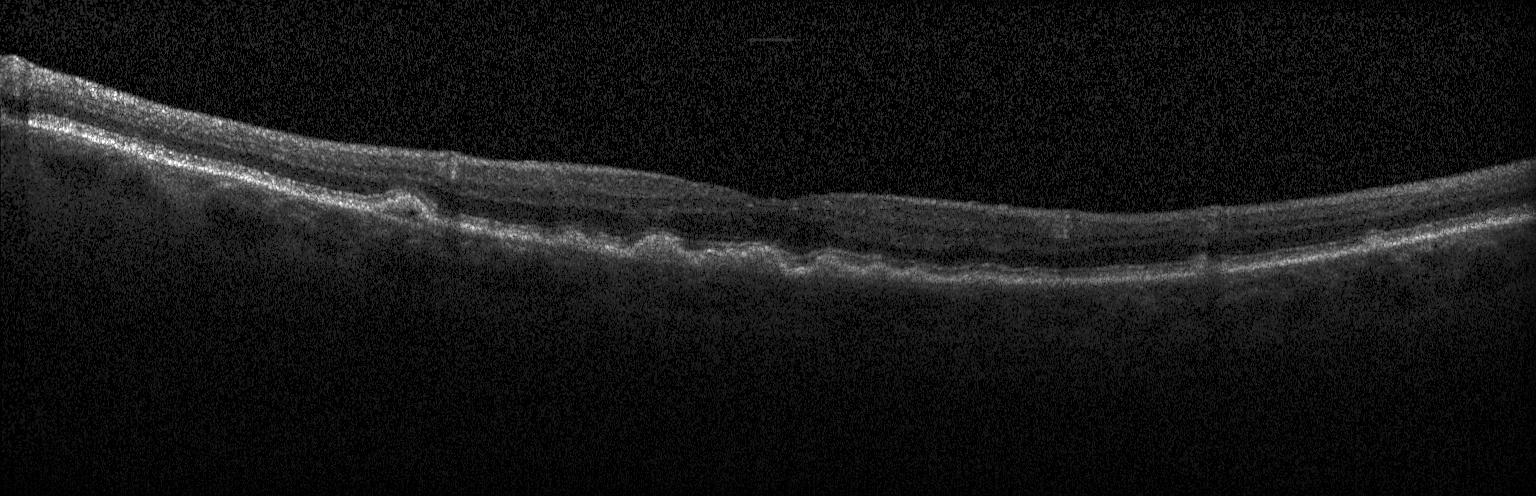

Retinal OCT B-scan. Spectral-domain optical coherence tomography
Diagnosis: multiple drusen.